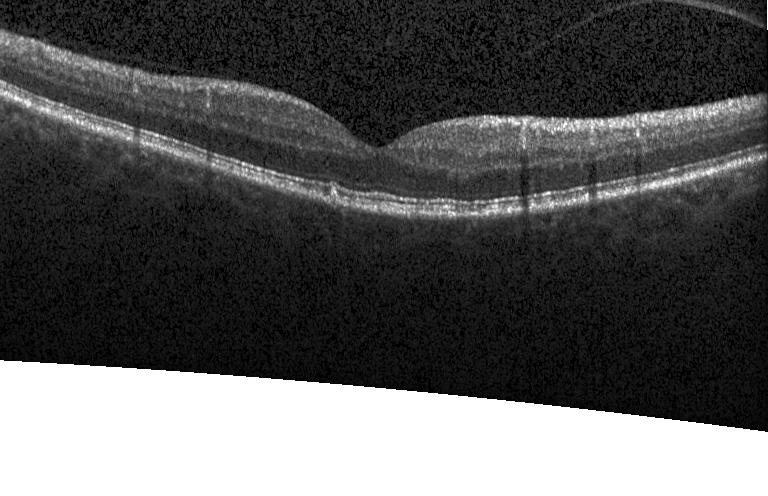
Spectral-domain OCT. OCT line scan. Instrument: Heidelberg Spectralis. OCT finding: drusen.